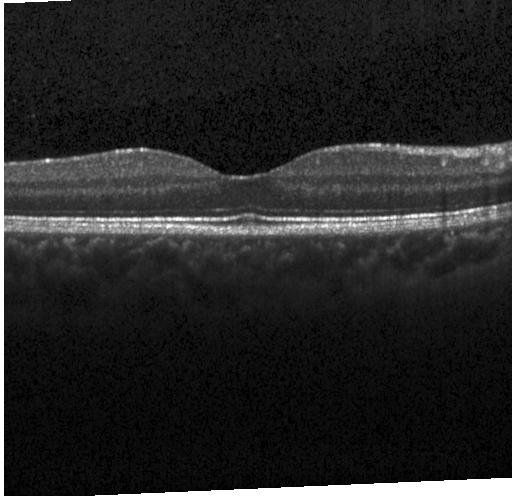

The scan shows no evidence of choroidal neovascularization, diabetic macular edema, or drusen.